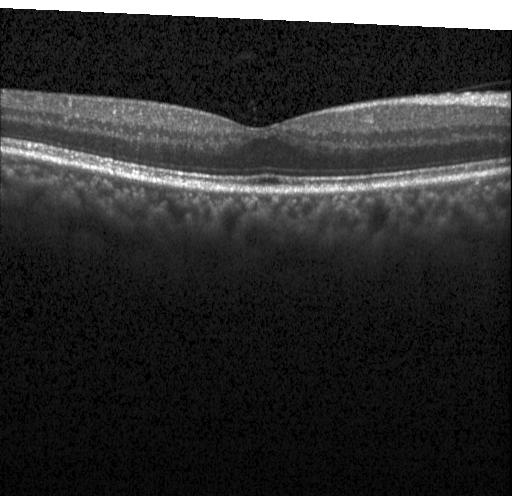
Diagnosis: neither choroidal neovascularization, diabetic macular edema, nor drusen.